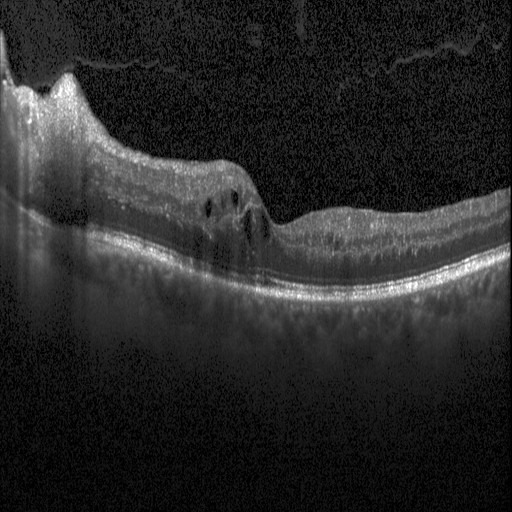

OCT line scan, through the macula, acquired on a Heidelberg Spectralis, spectral-domain optical coherence tomography — Impression: diabetic macular edema.